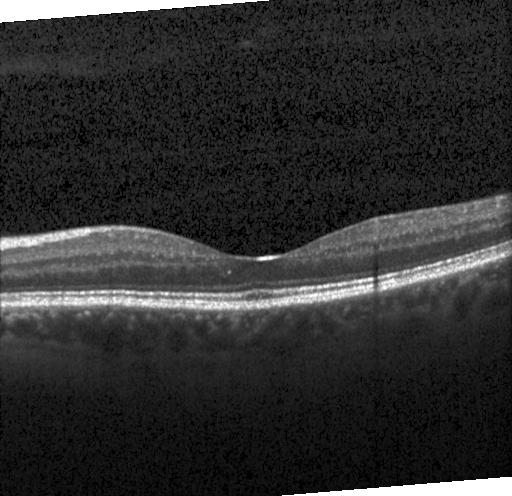 Instrument: Heidelberg Spectralis, OCT B-scan, spectral-domain OCT, through the macula. Diagnosis: no evidence of choroidal neovascularization, diabetic macular edema, or drusen.